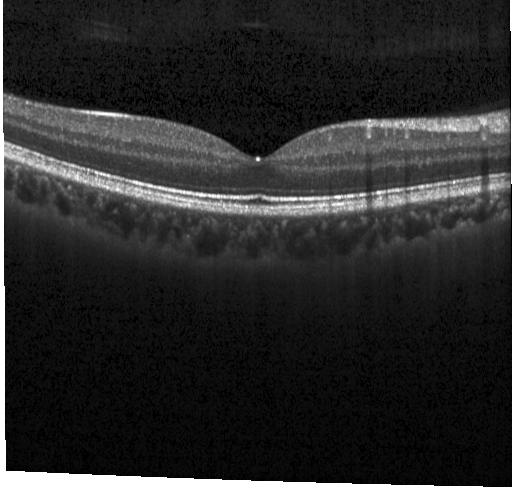
Retinal OCT cross-section — This B-scan demonstrates no evidence of CNV, DME, or drusen.